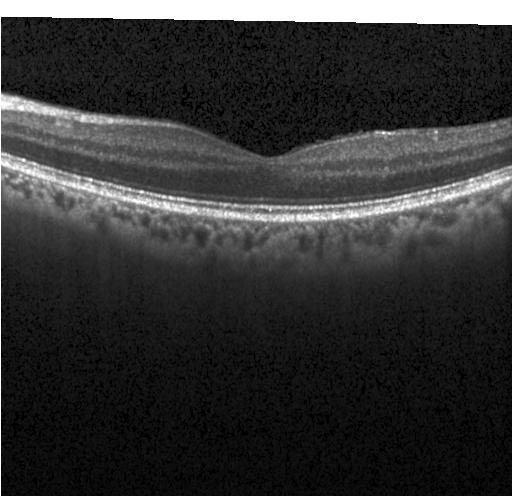 Through the macula; optical coherence tomography scan. Dx: neither choroidal neovascularization, diabetic macular edema, nor drusen.